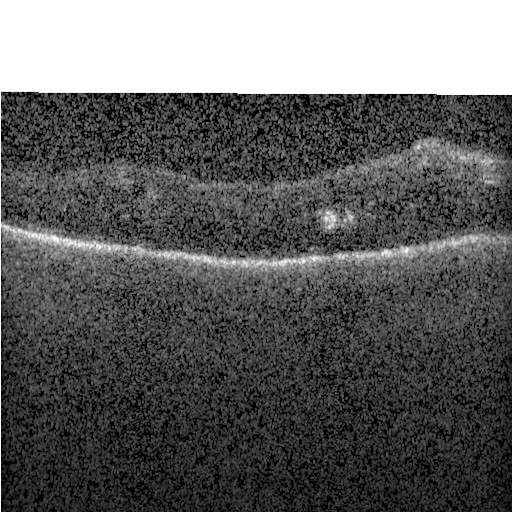

Optical coherence tomography B-scan — Macular OCT: DME.